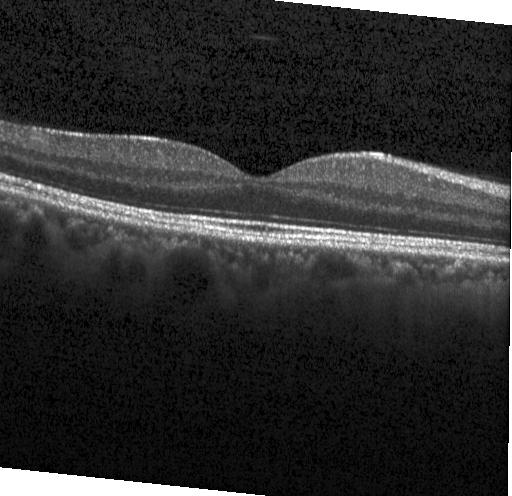
Centered on the fovea, OCT B-scan, instrument: Heidelberg Spectralis.
Impression: no CNV, DME, or drusen.